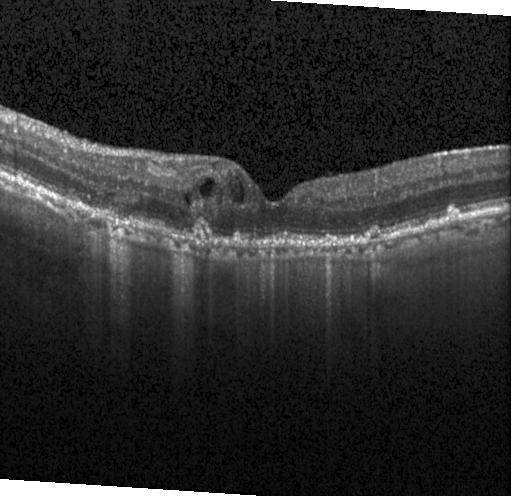

Heidelberg Spectralis. OCT B-scan. Fovea-centered — OCT finding: choroidal neovascularization (CNV).